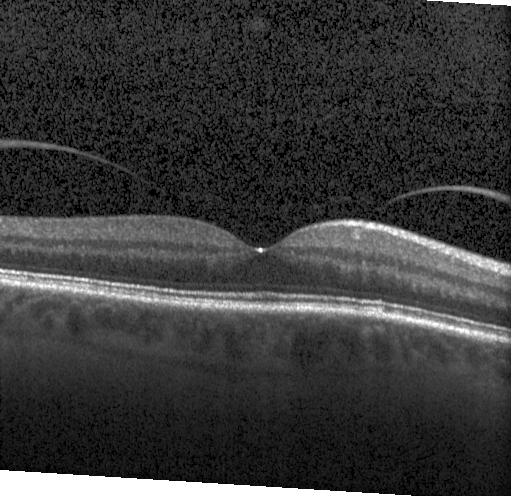 Heidelberg Spectralis, spectral-domain OCT, retinal OCT B-scan, through the macula — Dx: neither CNV, DME, nor drusen.